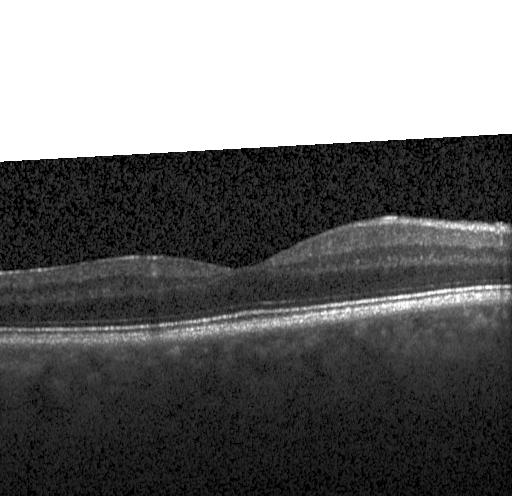
Dx: no choroidal neovascularization, diabetic macular edema, or drusen.